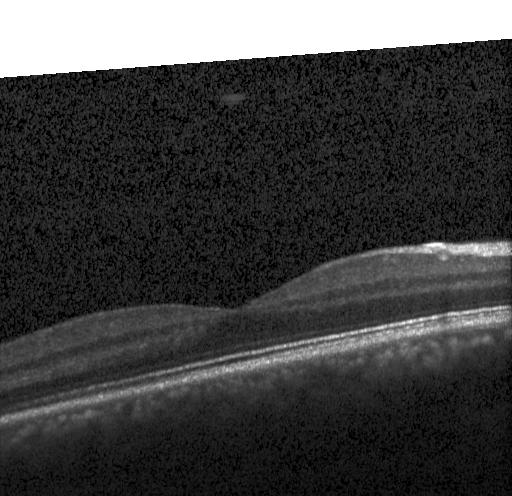
Retinal OCT B-scan — Impression: no choroidal neovascularization, diabetic macular edema, or drusen.